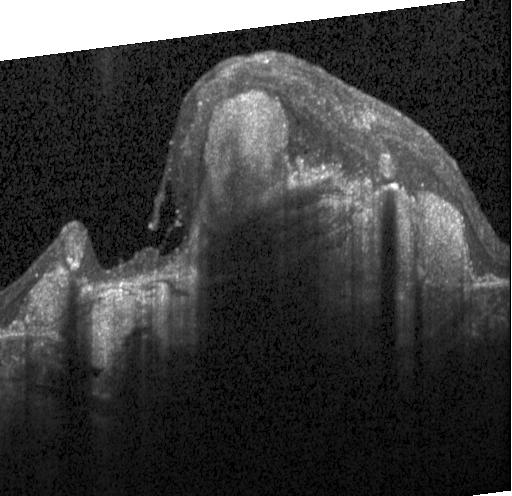
Retinal OCT cross-section showing a choroidal neovascular membrane.